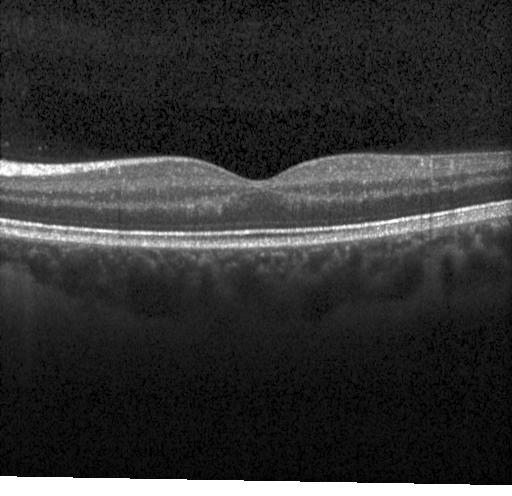
Optical coherence tomography B-scan. Impression: no choroidal neovascularization, diabetic macular edema, or drusen.